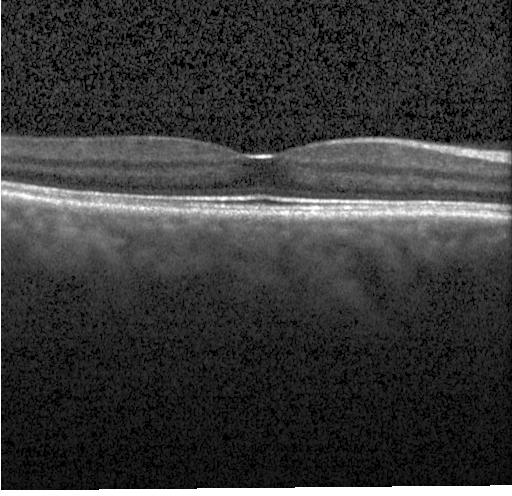
Retinal OCT B-scan, Heidelberg Spectralis OCT system, spectral-domain optical coherence tomography, centered on the fovea. Diagnosis: no choroidal neovascularization, diabetic macular edema, or drusen.